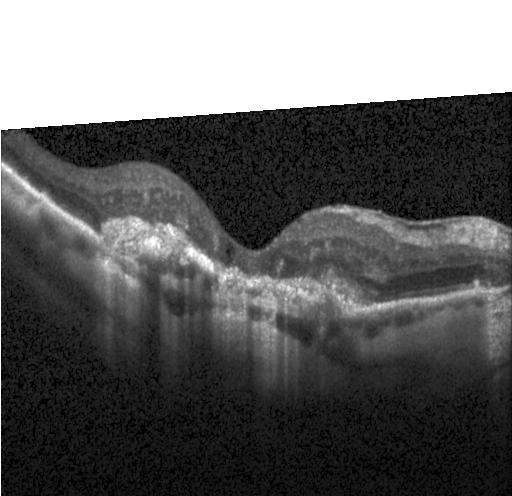
Optical coherence tomography B-scan. Diagnosis: a choroidal neovascular membrane.